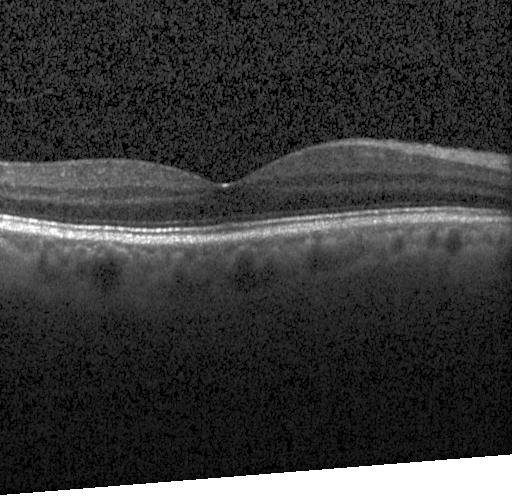

Diagnosis: no choroidal neovascularization, diabetic macular edema, or drusen.